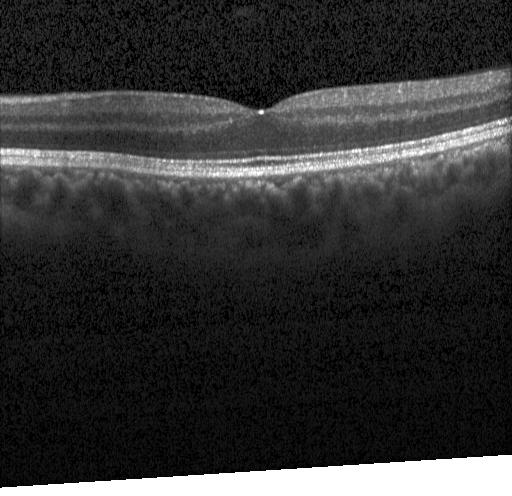
Horizontal scan through the fovea, OCT line scan.
Diagnosis: no evidence of choroidal neovascularization, diabetic macular edema, or drusen.